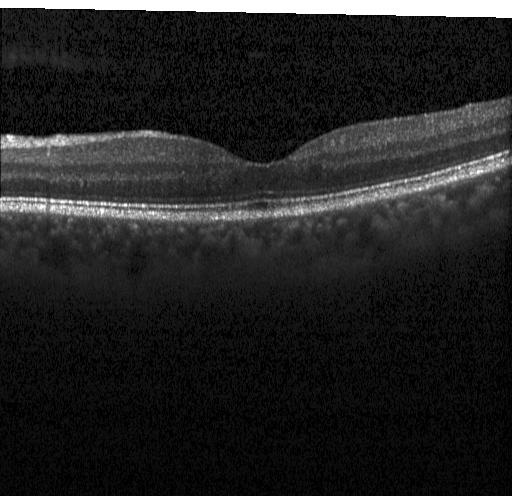 Impression: neither choroidal neovascularization, diabetic macular edema, nor drusen.